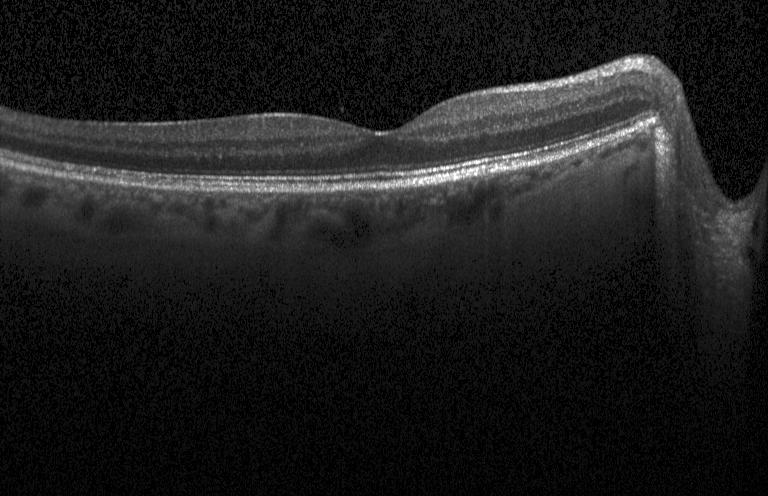
Optical coherence tomography B-scan
Assessment: no choroidal neovascularization, no diabetic macular edema, and no drusen.